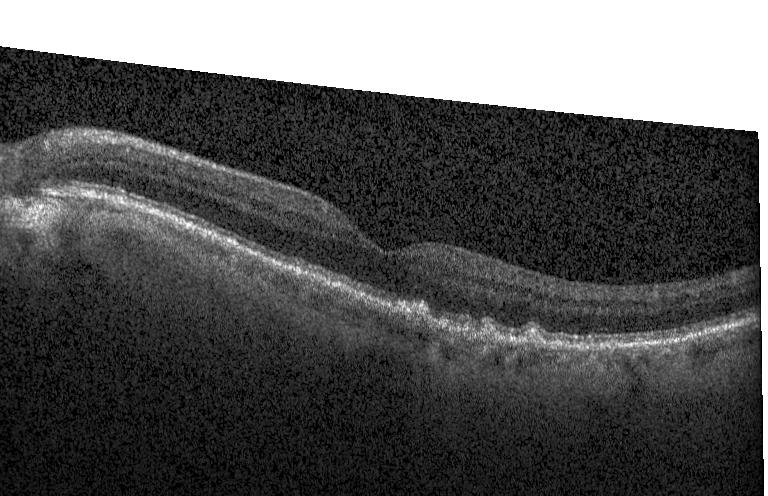

Retinal OCT B-scan. Fovea-centered. Drusen.